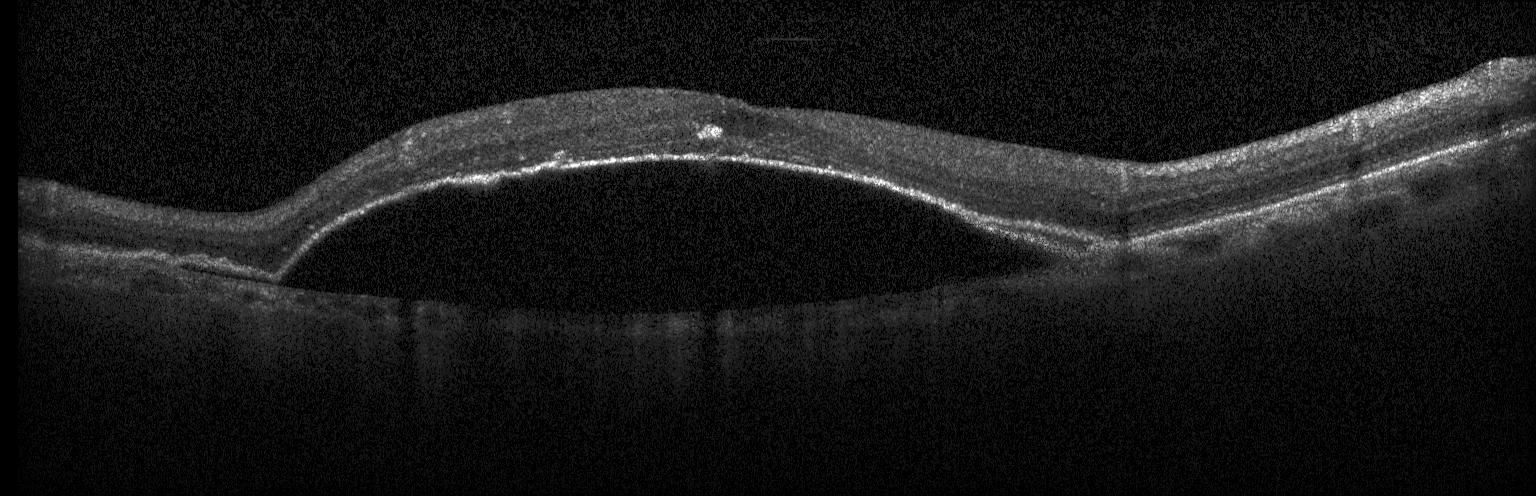
Retinal OCT B-scan; macular scan — Dx: a choroidal neovascular membrane.